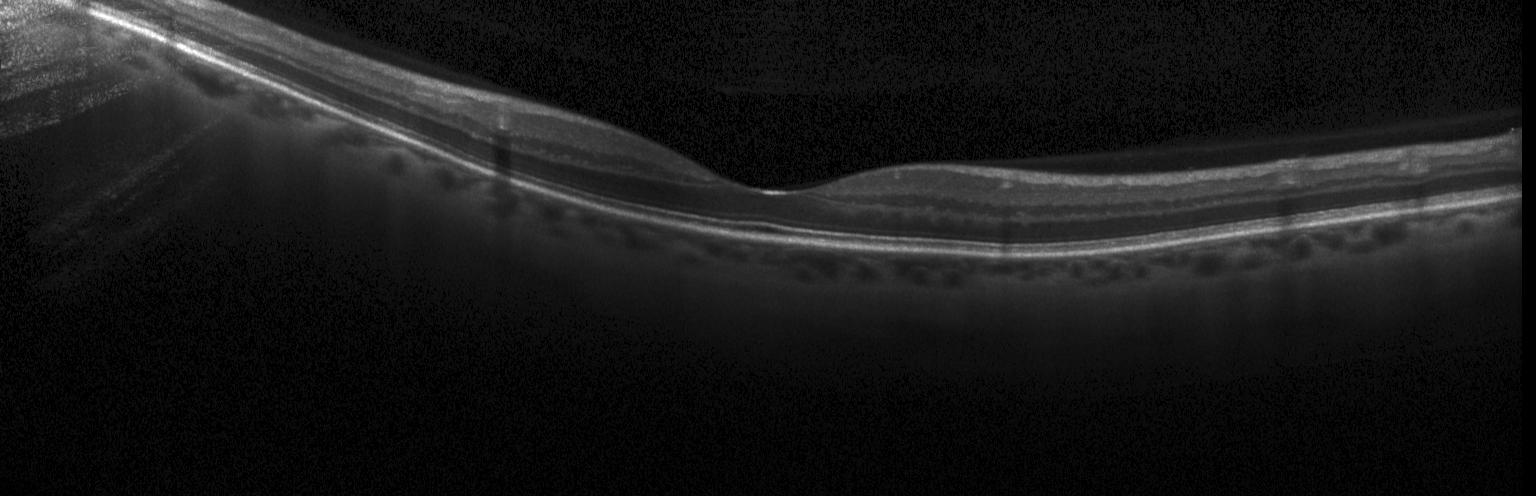 Retinal OCT B-scan, horizontal scan through the fovea. Diagnosis: no choroidal neovascularization, no diabetic macular edema, and no drusen.